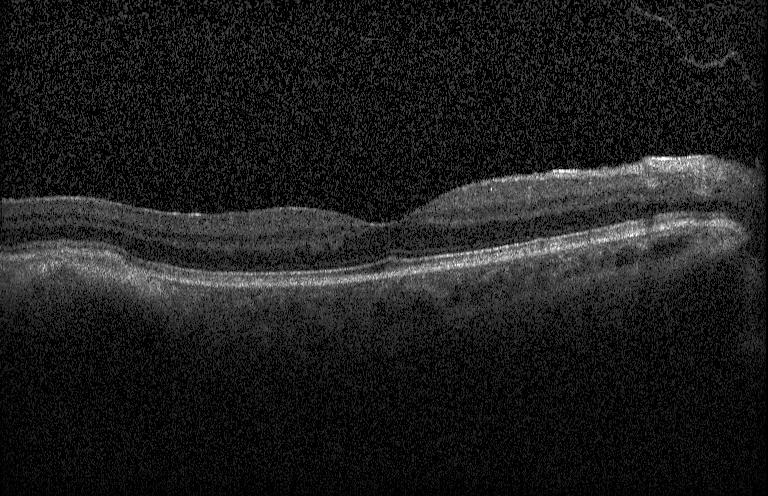

OCT line scan, instrument: Heidelberg Spectralis. Assessment: choroidal neovascularization (CNV).